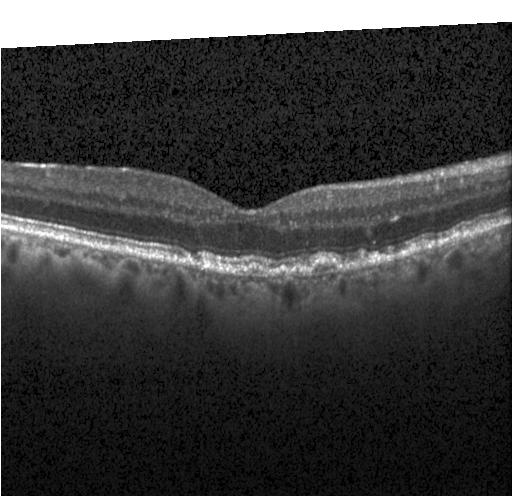

Impression: multiple drusen.